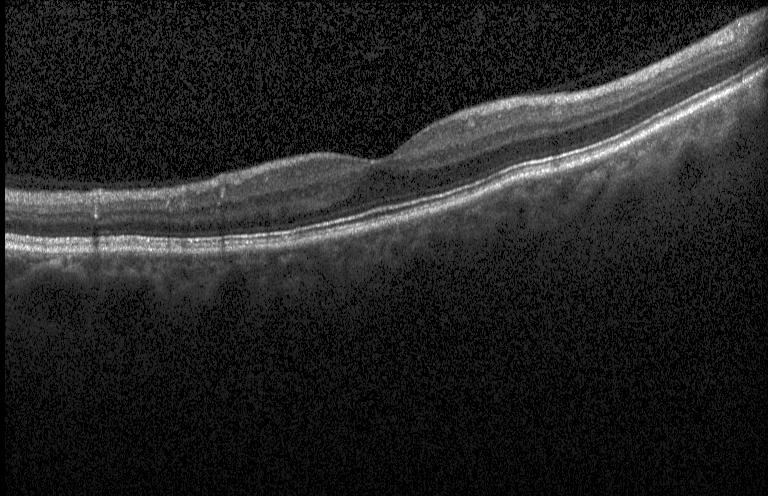

Finding: no choroidal neovascularization, no diabetic macular edema, and no drusen.